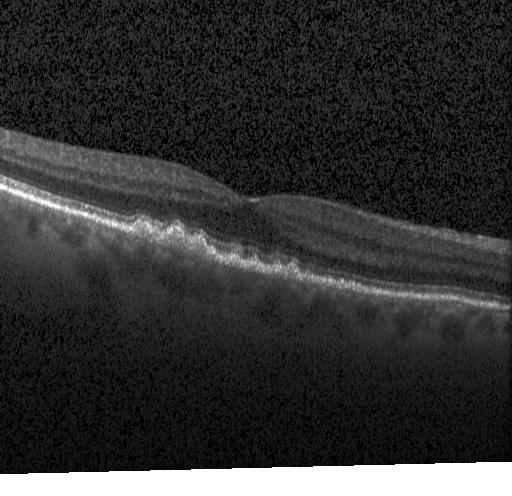 Instrument: Heidelberg Spectralis; optical coherence tomography scan — Macular OCT: drusen.